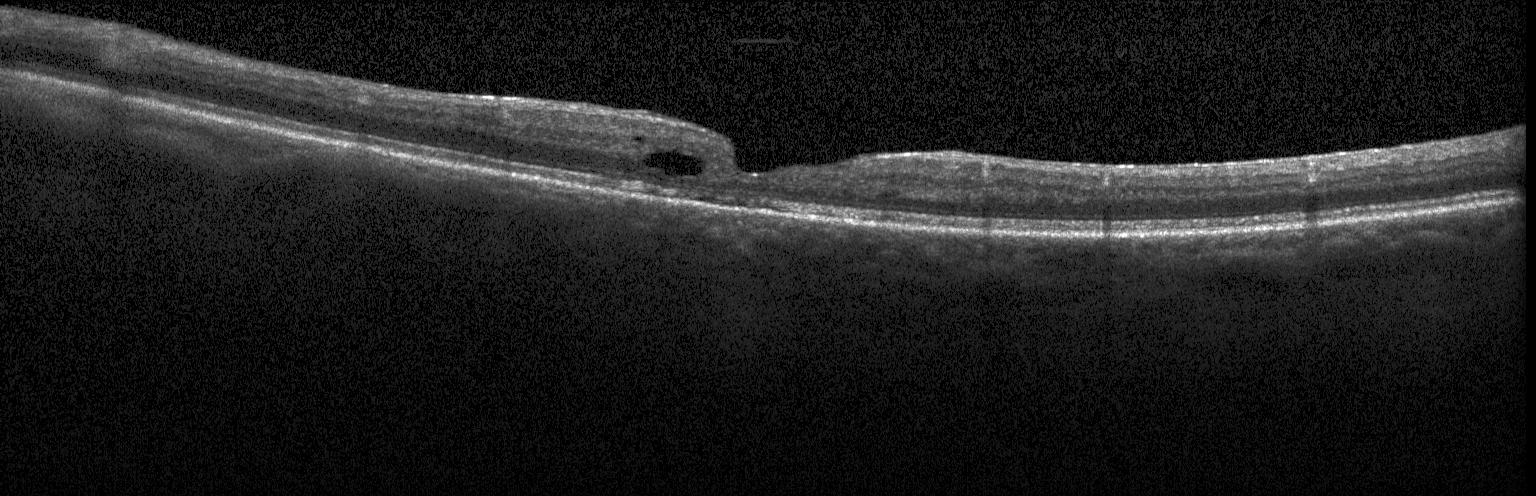

SD-OCT · retinal OCT B-scan · fovea-centered
Macular OCT: DME.